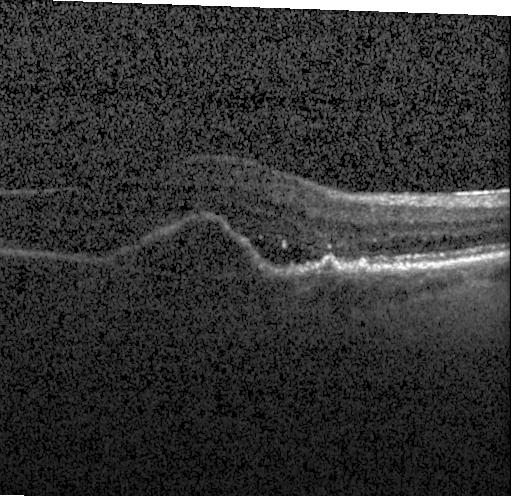
Spectral-domain optical coherence tomography · instrument: Heidelberg Spectralis · optical coherence tomography B-scan · macular scan — This B-scan demonstrates CNV.